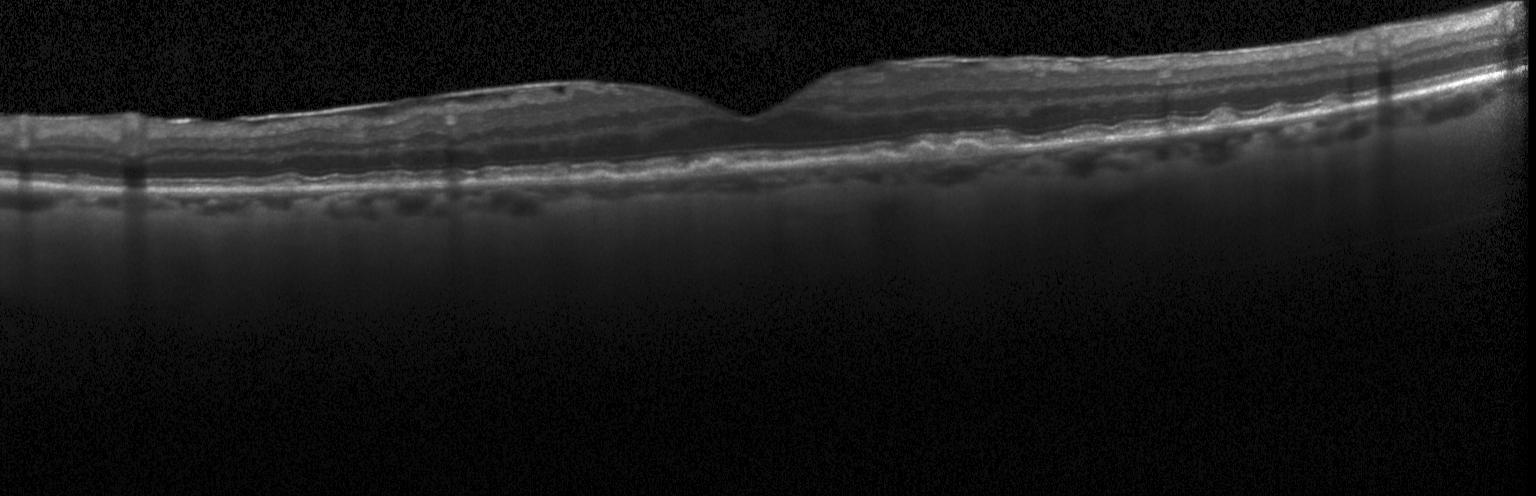 Retinal OCT B-scan; Heidelberg Spectralis
Impression: multiple drusen.